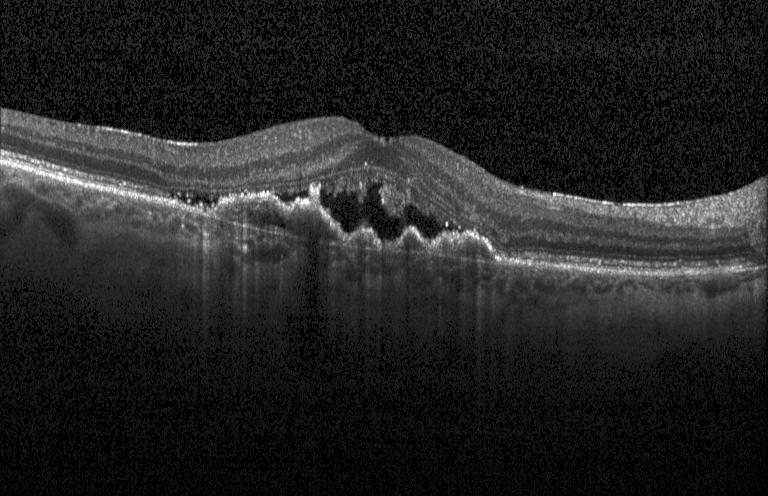

Retinal OCT B-scan, spectral-domain optical coherence tomography. Finding: choroidal neovascularization (CNV).